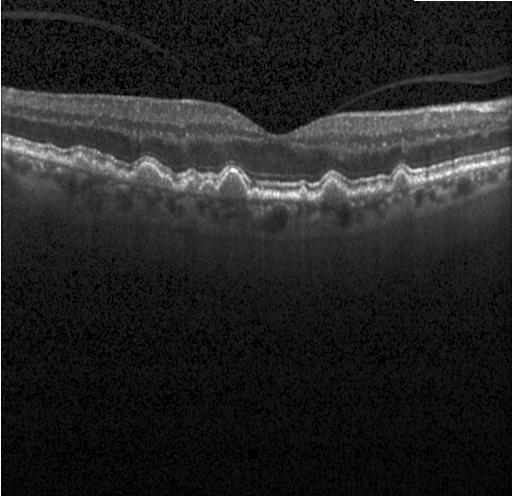 OCT B-scan, centered on the fovea
Assessment: sub-RPE drusenoid deposits.